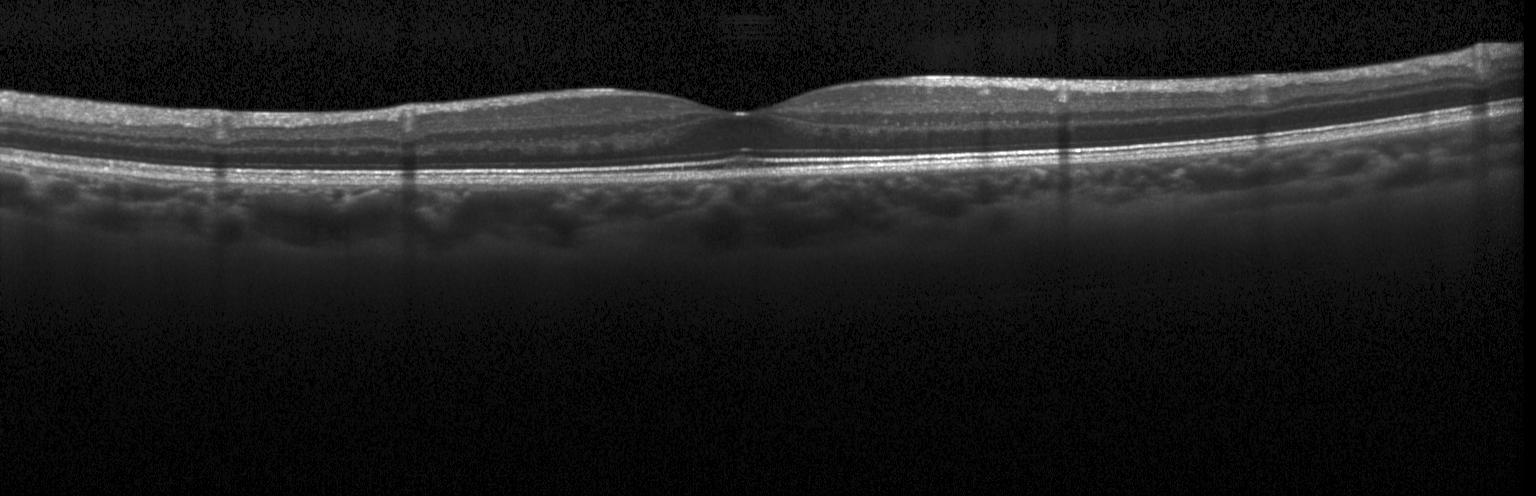 OCT line scan, Heidelberg Spectralis OCT system — Assessment: neither choroidal neovascularization, diabetic macular edema, nor drusen.